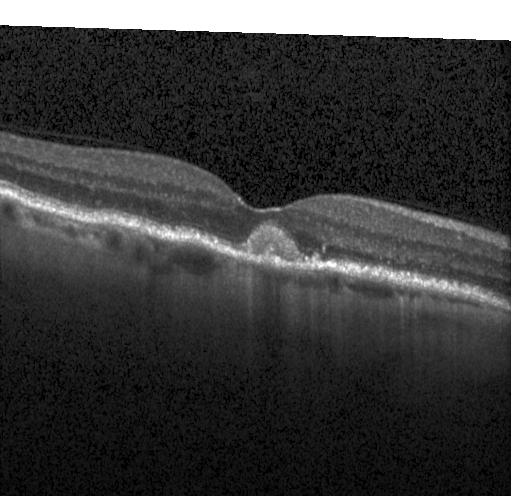

OCT B-scan
The scan shows drusen.